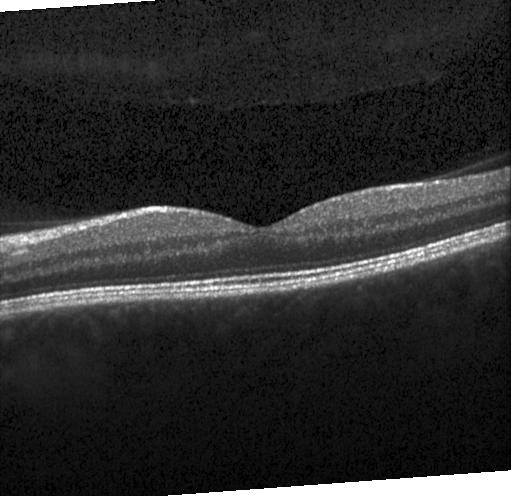 Heidelberg Spectralis OCT system. Centered on the fovea. Optical coherence tomography B-scan. Spectral-domain OCT. Finding: neither CNV, DME, nor drusen.